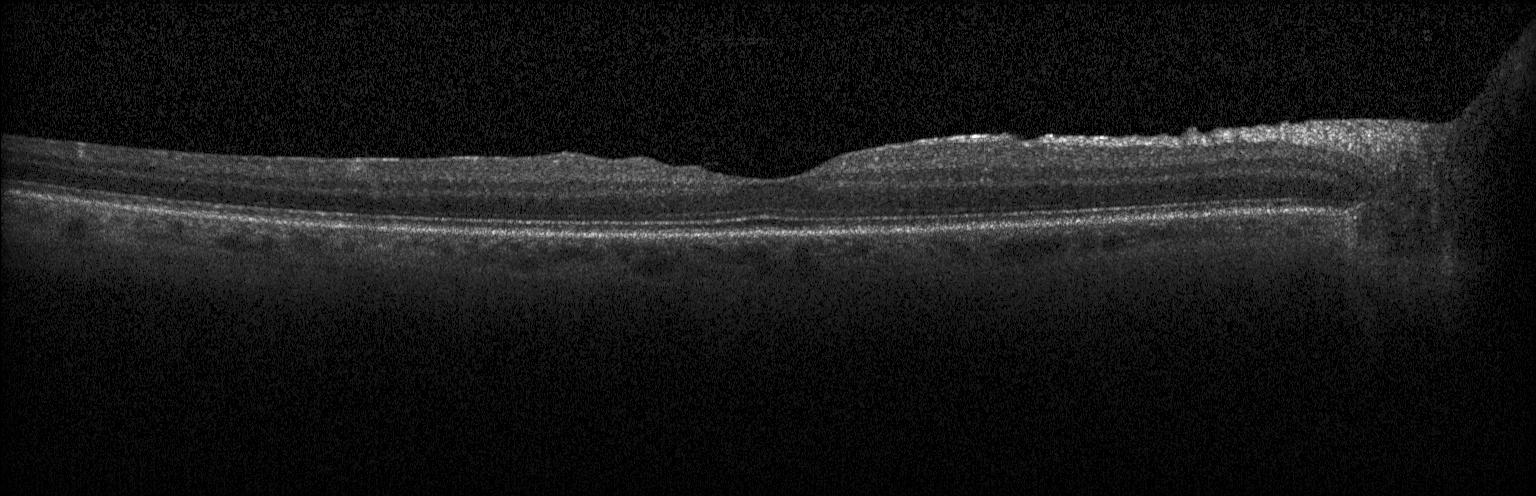

Heidelberg Spectralis · retinal OCT B-scan · horizontal scan through the fovea.
Macular OCT: neither choroidal neovascularization, diabetic macular edema, nor drusen.